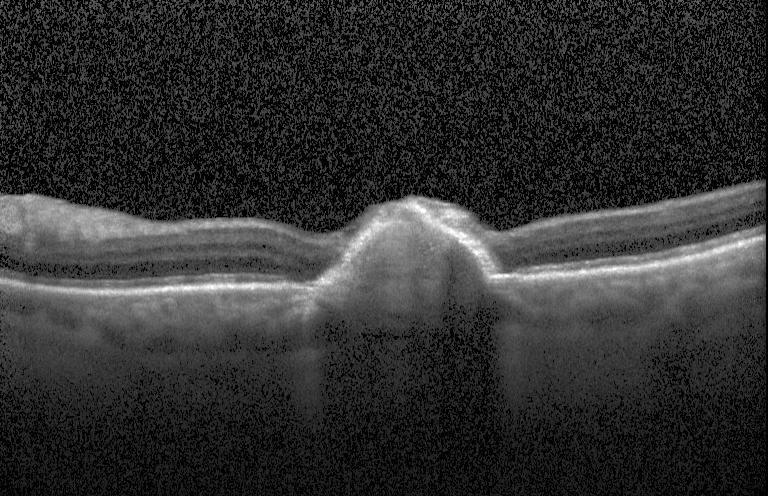 This B-scan demonstrates choroidal neovascularization (CNV).